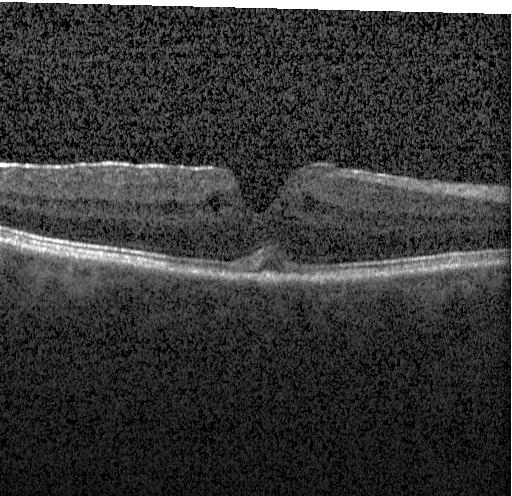

Retinal OCT B-scan
Impression: diabetic macular edema.